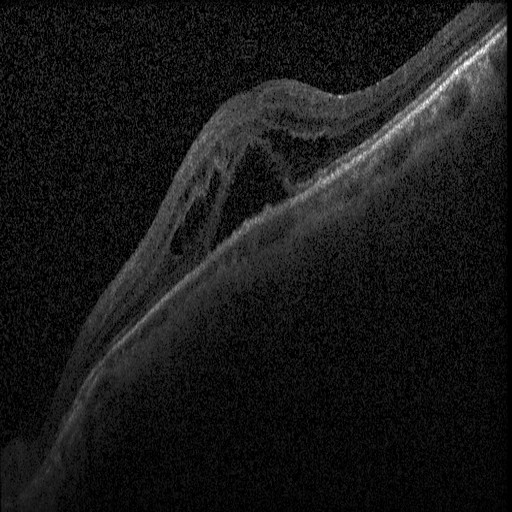
OCT B-scan; through the macula
This B-scan demonstrates diabetic macular edema.